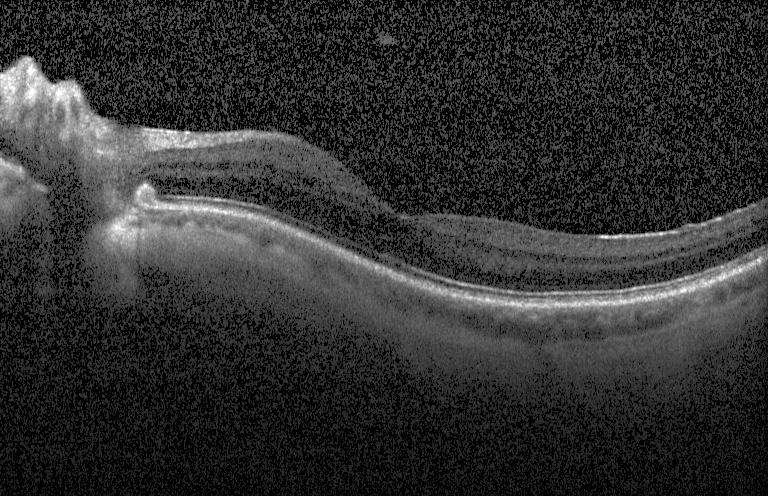

Spectral-domain optical coherence tomography. Heidelberg Spectralis. OCT line scan. Centered on the fovea
Impression: drusen.